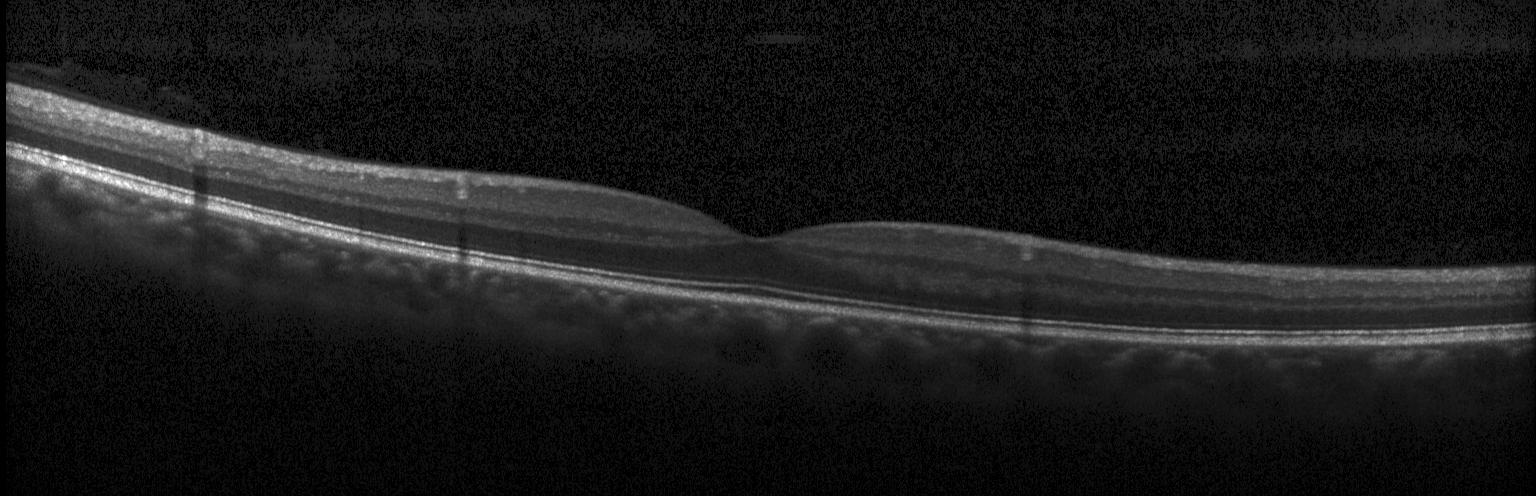 OCT line scan. Diagnosis: neither CNV, DME, nor drusen.